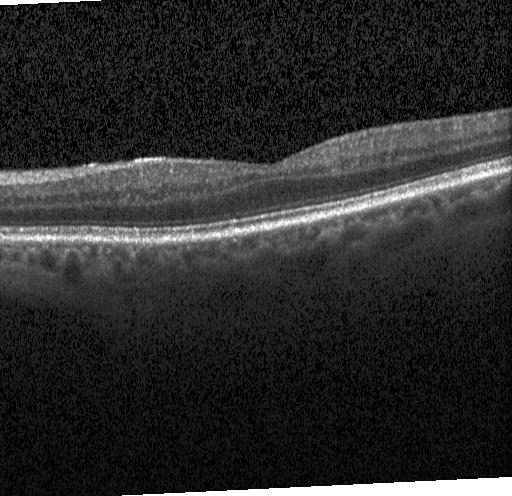 Spectral-domain optical coherence tomography. Instrument: Heidelberg Spectralis. Retinal OCT B-scan
Dx: no evidence of choroidal neovascularization, diabetic macular edema, or drusen.